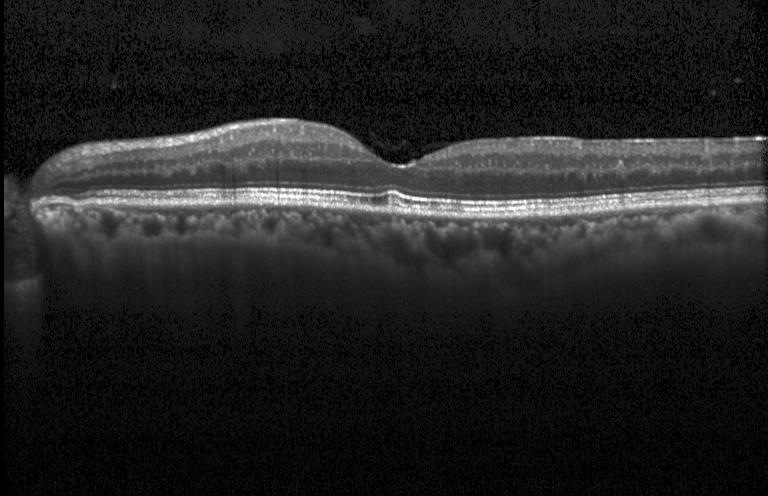

The scan shows no CNV, no DME, and no drusen.